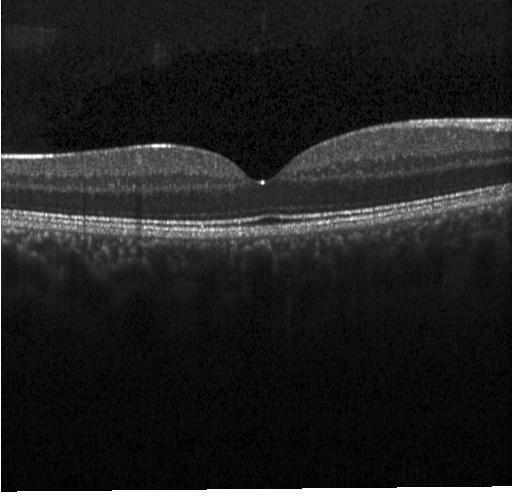

Heidelberg Spectralis. Horizontal scan through the fovea. SD-OCT. OCT line scan.
Macular OCT: no CNV, DME, or drusen.